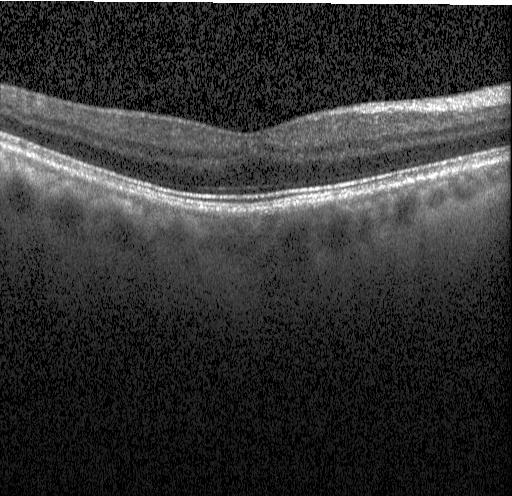
Impression: no choroidal neovascularization, no diabetic macular edema, and no drusen.